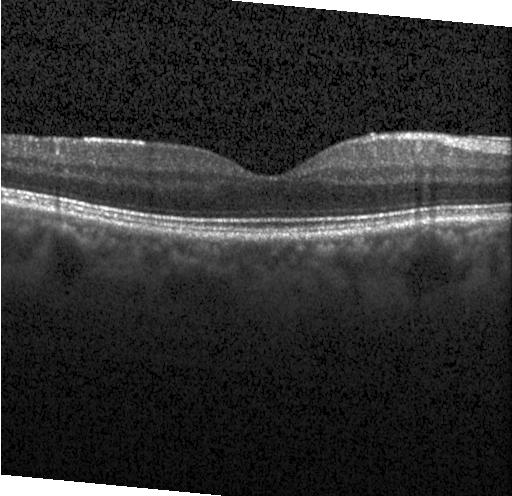

This B-scan demonstrates no CNV, DME, or drusen.